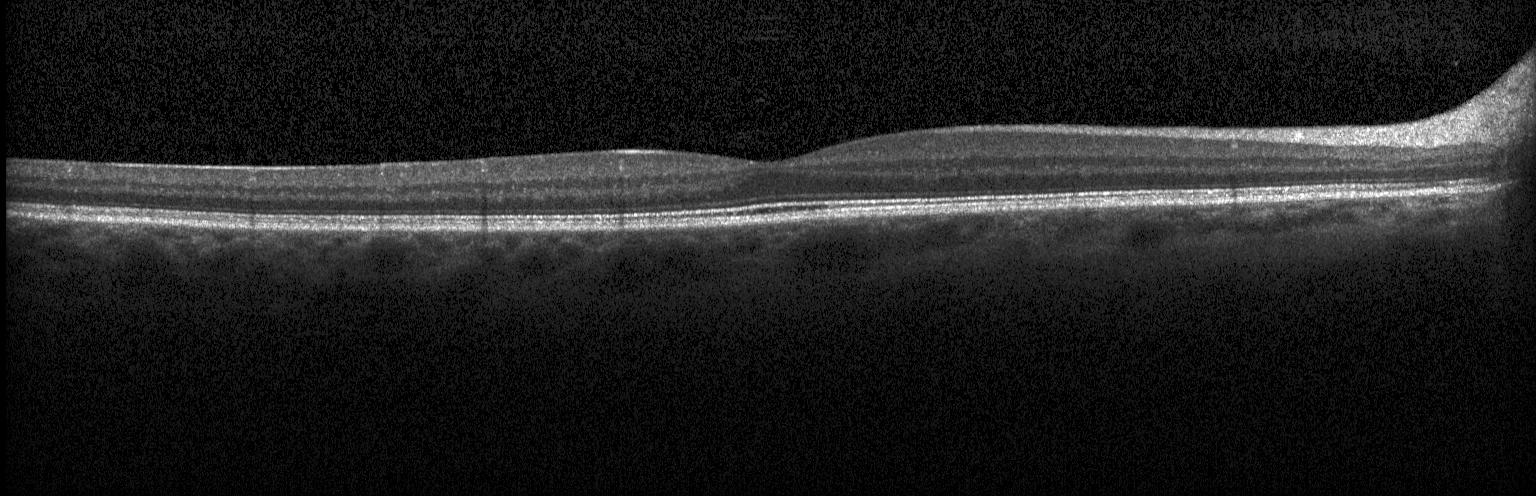 Macular OCT: no choroidal neovascularization, no diabetic macular edema, and no drusen.